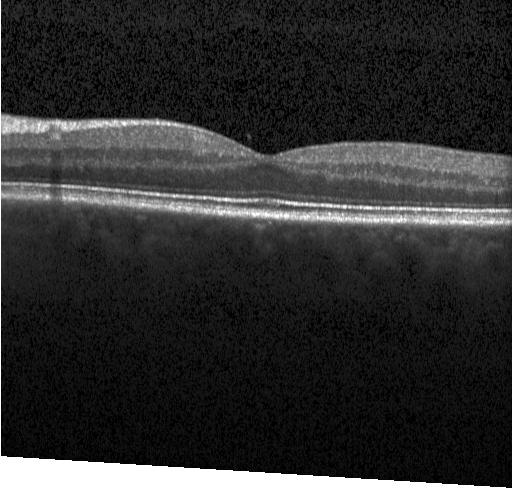
Optical coherence tomography B-scan. SD-OCT.
This B-scan demonstrates neither CNV, DME, nor drusen.